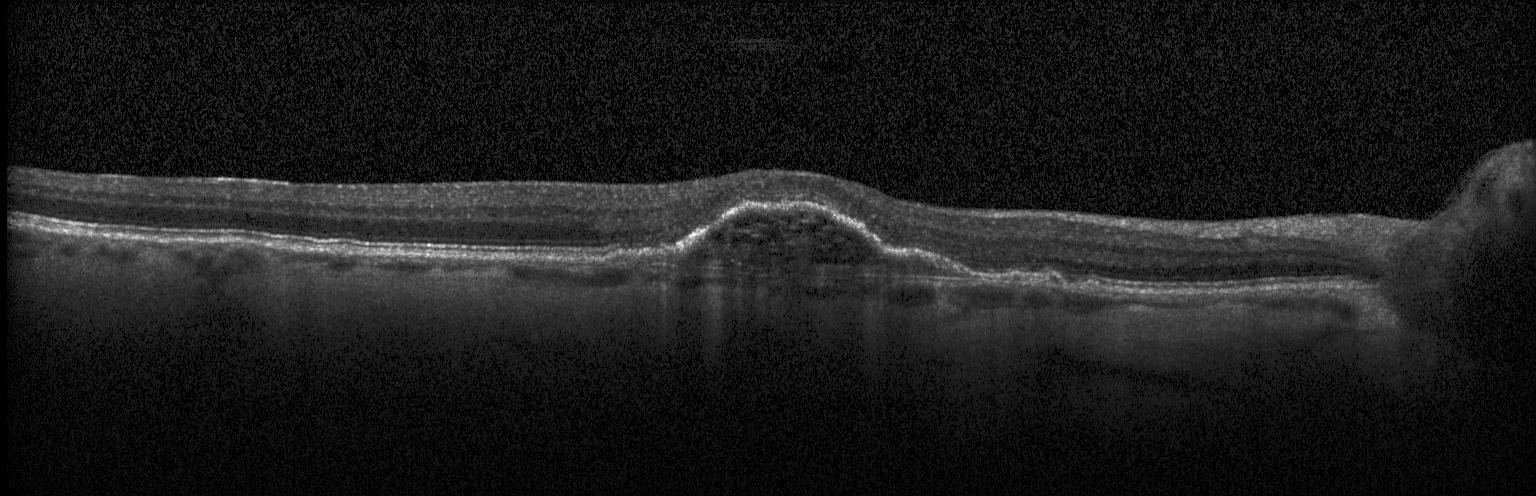
SD-OCT; retinal OCT B-scan — Impression: a choroidal neovascular membrane.